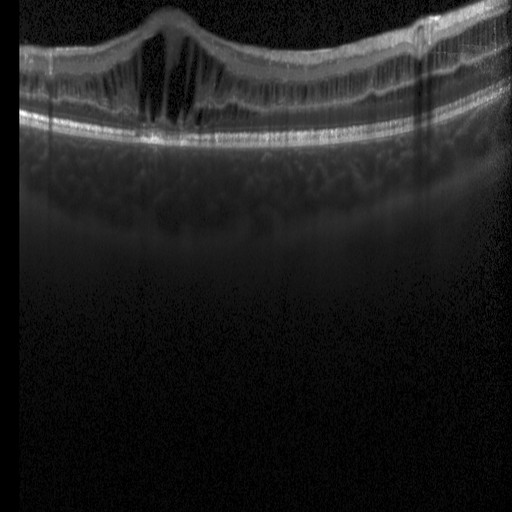 Instrument: Heidelberg Spectralis, spectral-domain OCT, optical coherence tomography B-scan, through the macula. Dx: DME.